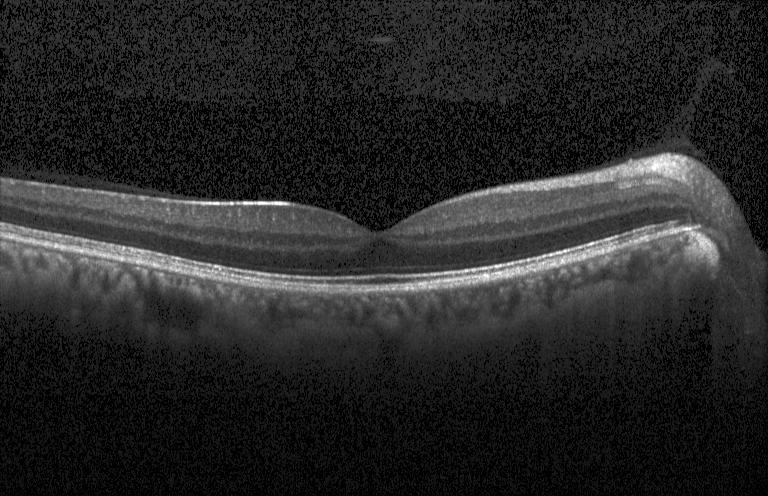

Assessment: no CNV, DME, or drusen.